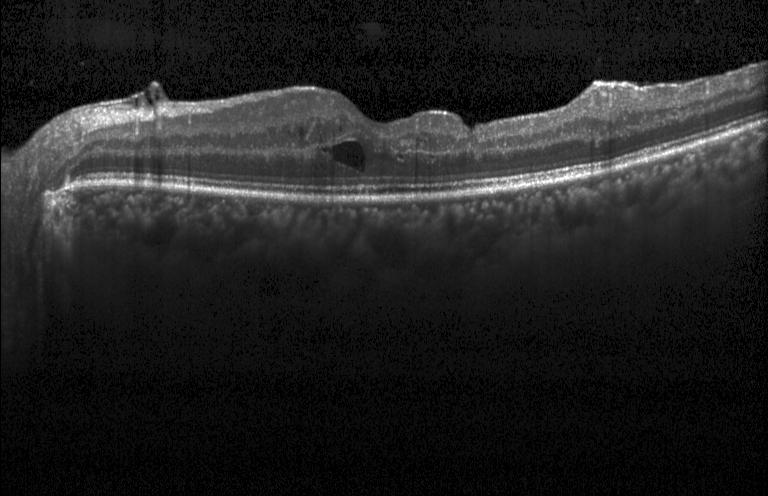 Retinal OCT B-scan.
Finding: diabetic macular edema.